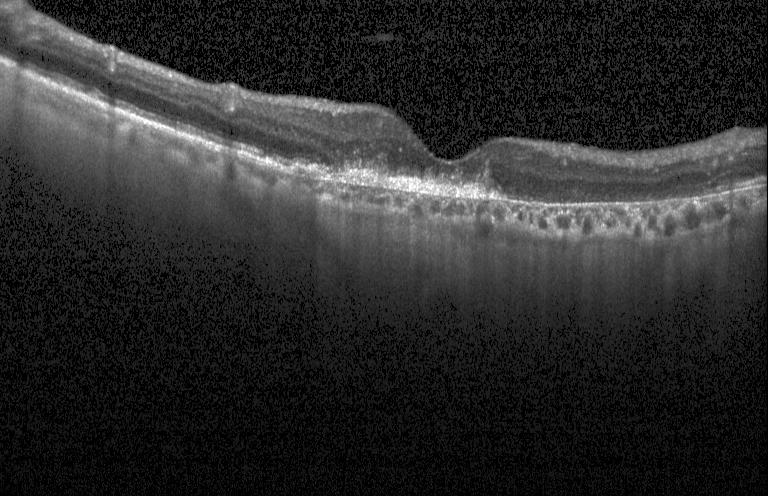 Optical coherence tomography B-scan, Heidelberg Spectralis OCT system, through the macula
Choroidal neovascularization.